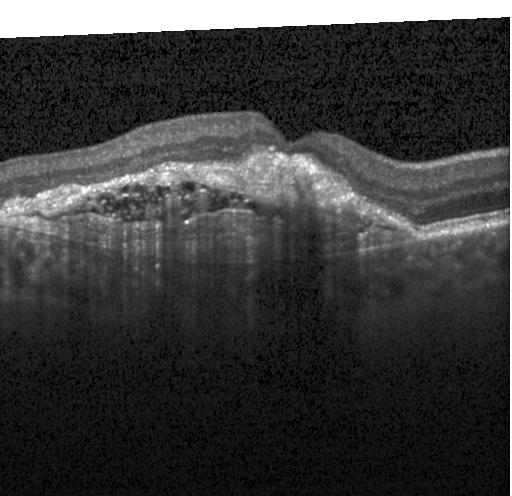
Retinal OCT cross-section, spectral-domain OCT, centered on the fovea
The scan shows choroidal neovascularization (CNV).